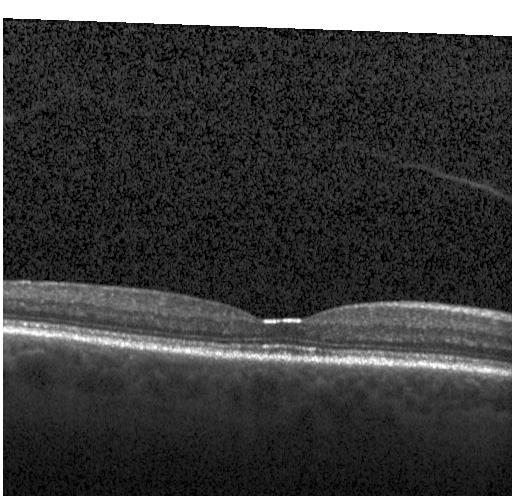
Fovea-centered · OCT line scan · instrument: Heidelberg Spectralis · spectral-domain OCT. Finding: neither choroidal neovascularization, diabetic macular edema, nor drusen.